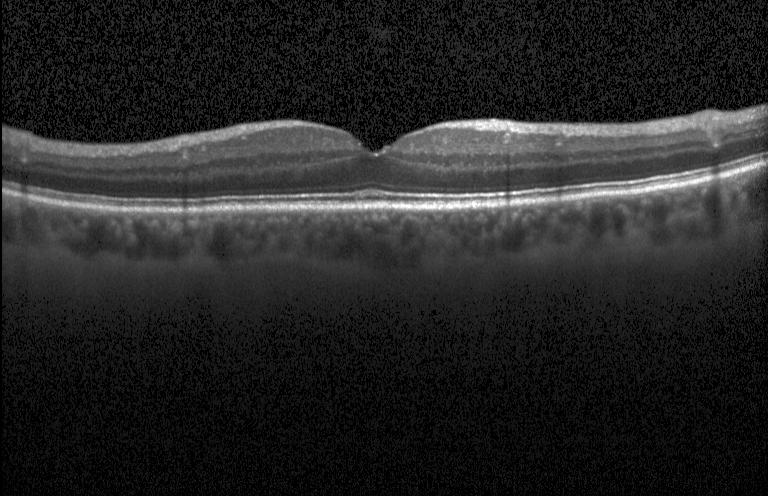

Macular OCT demonstrating no evidence of choroidal neovascularization, diabetic macular edema, or drusen.